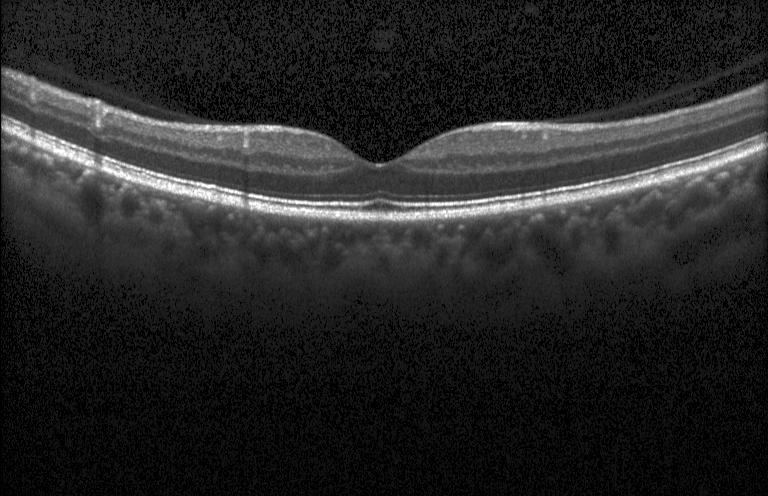

The scan shows no CNV, DME, or drusen.